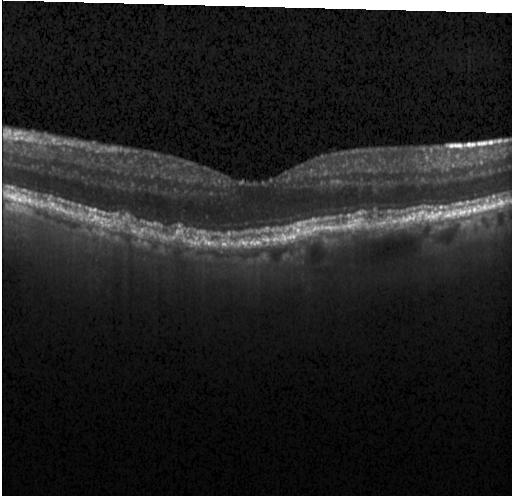 The scan shows multiple drusen.